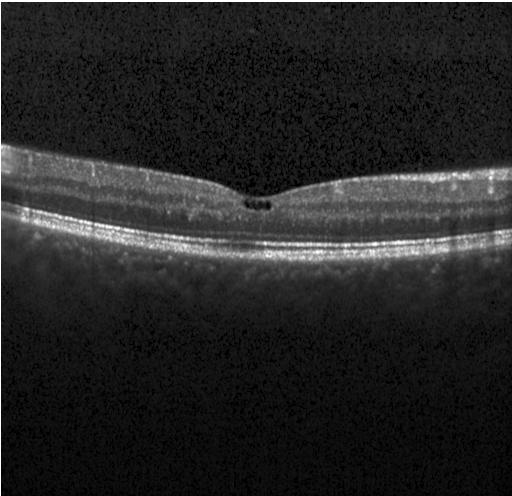

The scan shows diabetic macular edema (DME).